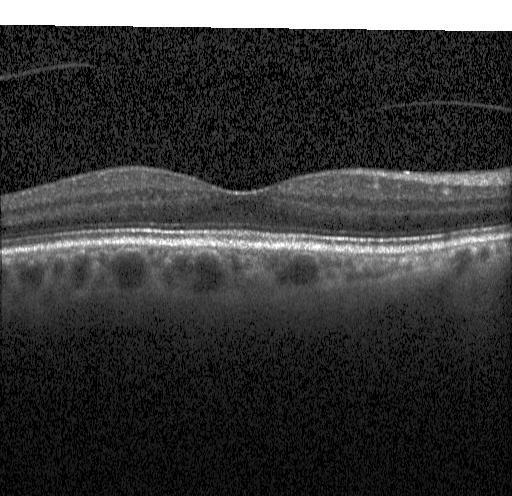
This B-scan demonstrates no evidence of choroidal neovascularization, diabetic macular edema, or drusen.